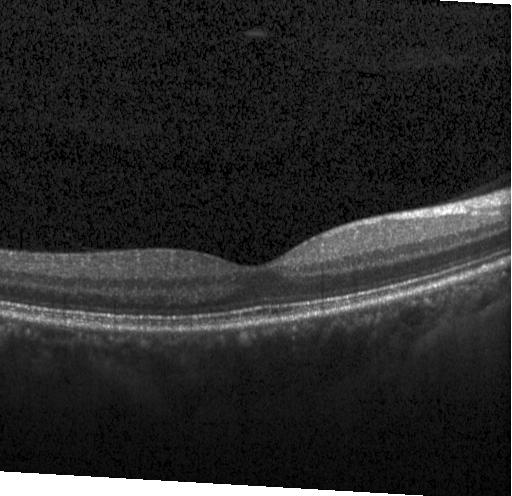
Optical coherence tomography B-scan; SD-OCT; instrument: Heidelberg Spectralis; through the macula. Dx: no choroidal neovascularization, no diabetic macular edema, and no drusen.